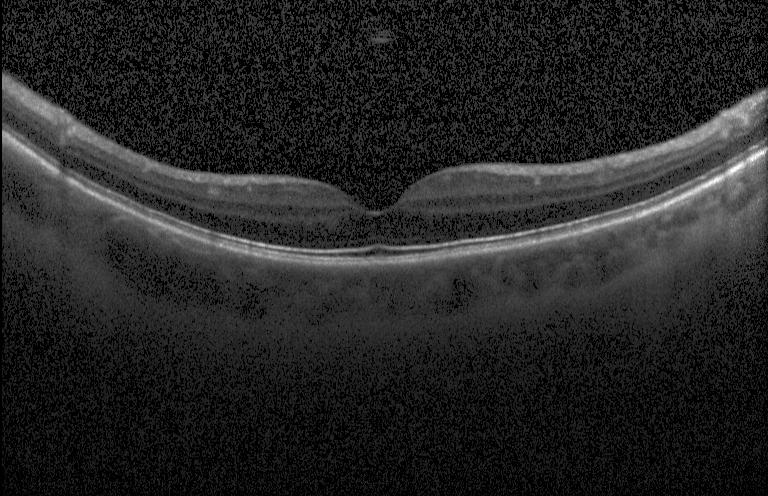

Optical coherence tomography B-scan. Finding: no evidence of choroidal neovascularization, diabetic macular edema, or drusen.